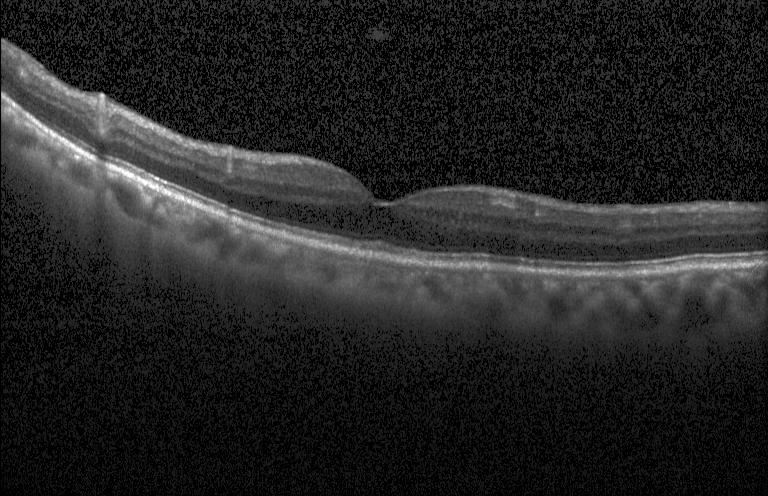

Optical coherence tomography B-scan; macular scan. Macular OCT: no evidence of choroidal neovascularization, diabetic macular edema, or drusen.